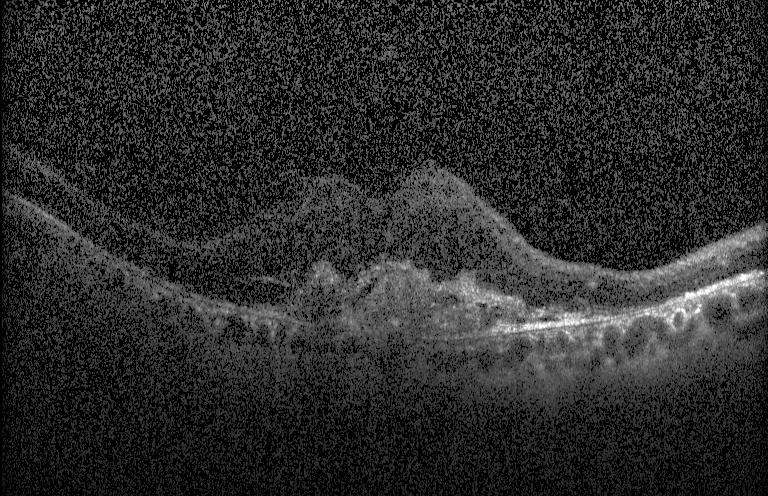 Optical coherence tomography B-scan, Heidelberg Spectralis, fovea-centered. Macular OCT: choroidal neovascularization.